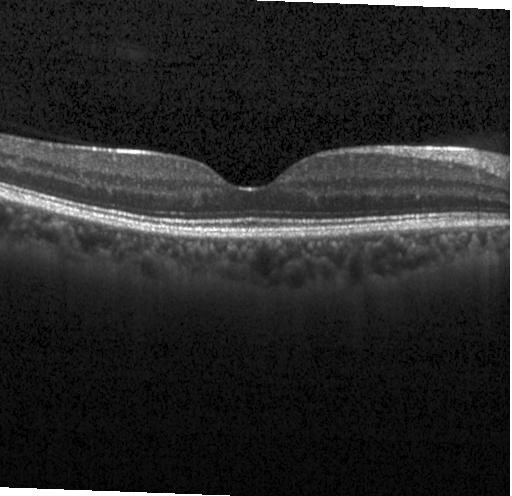
Optical coherence tomography B-scan.
OCT finding: no evidence of CNV, DME, or drusen.